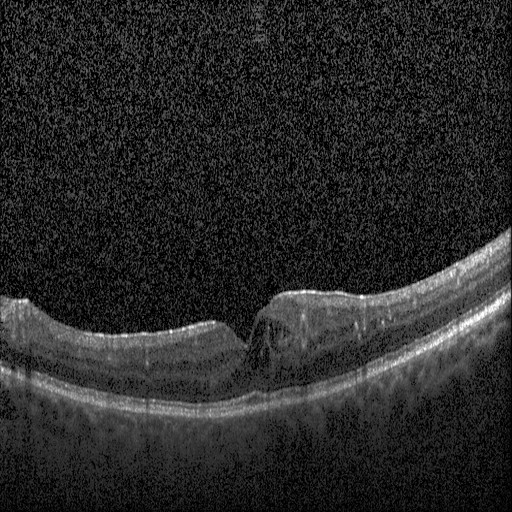 Through the macula. Optical coherence tomography scan.
Finding: diabetic macular edema (DME).